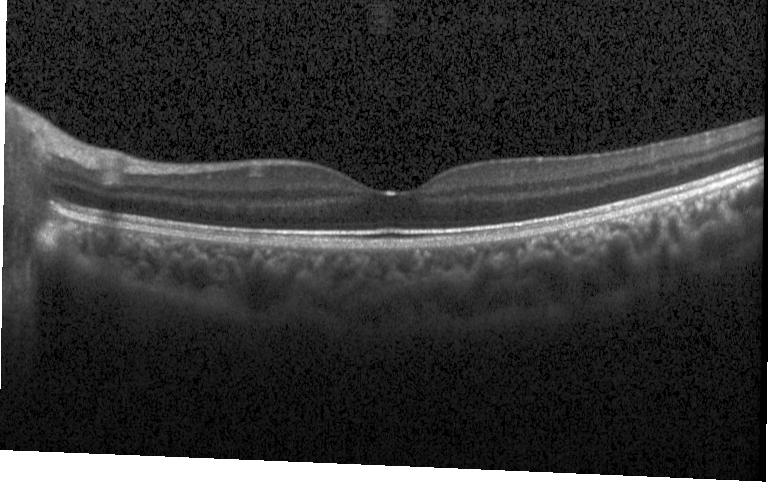

OCT B-scan, horizontal scan through the fovea, spectral-domain OCT, instrument: Heidelberg Spectralis
Macular OCT: no evidence of choroidal neovascularization, diabetic macular edema, or drusen.